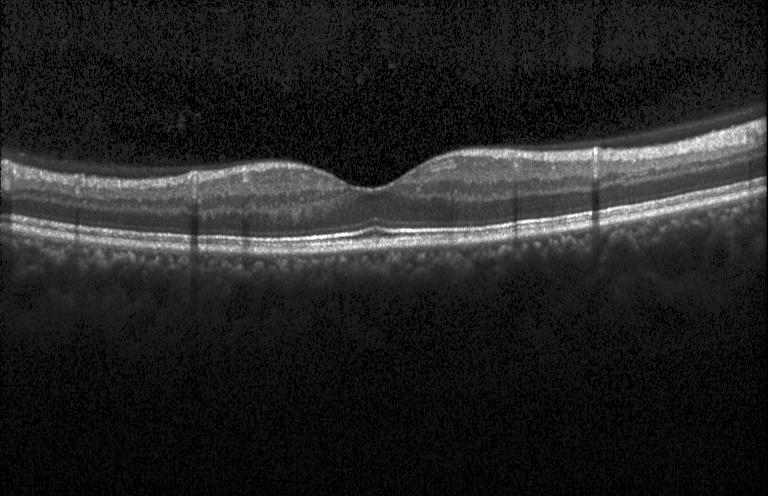 Horizontal scan through the fovea · OCT B-scan · Heidelberg Spectralis OCT system · spectral-domain optical coherence tomography.
Macular OCT: no choroidal neovascularization, no diabetic macular edema, and no drusen.